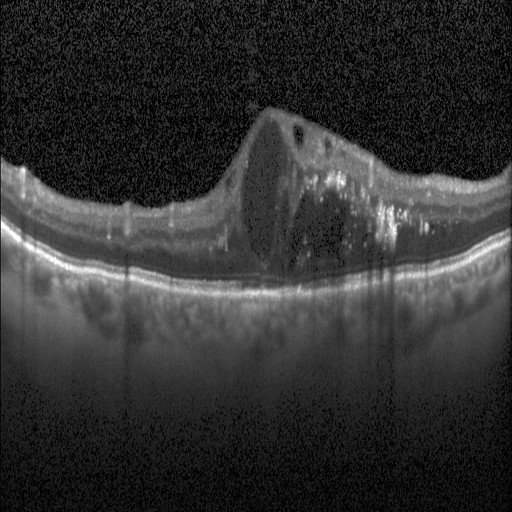

SD-OCT · Heidelberg Spectralis · optical coherence tomography scan · centered on the fovea
Diabetic macular edema.